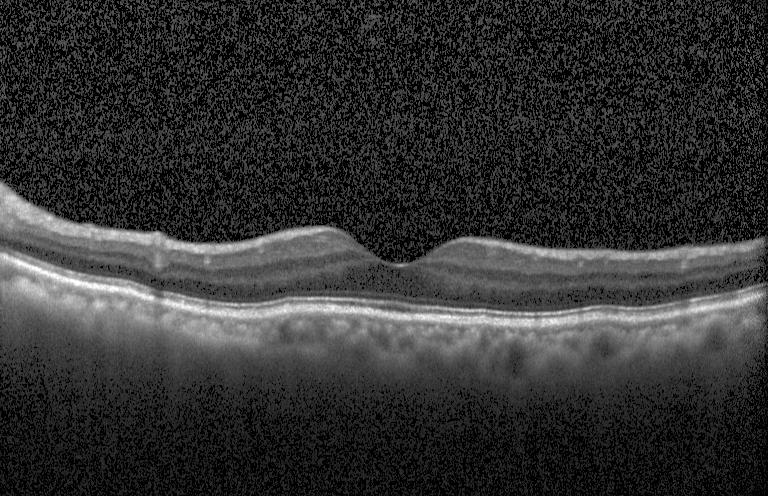

Diagnosis: no CNV, no DME, and no drusen.